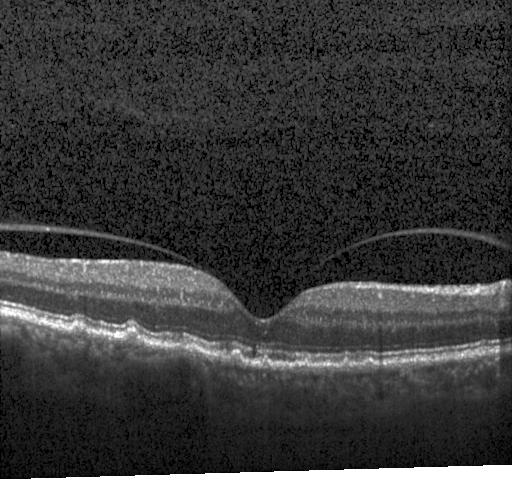 Dx: drusen.